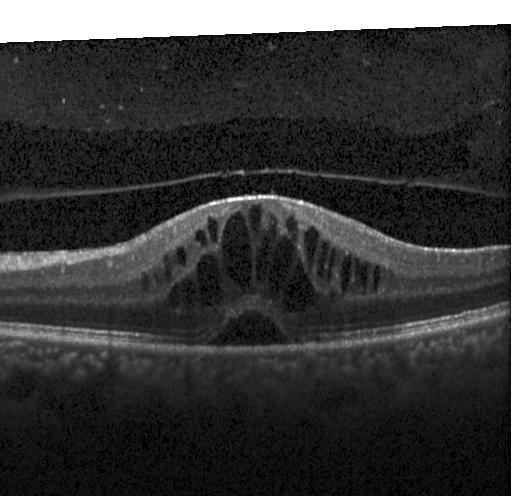 Spectral-domain optical coherence tomography. Retinal OCT cross-section. Macular scan — Diagnosis: diabetic macular edema.